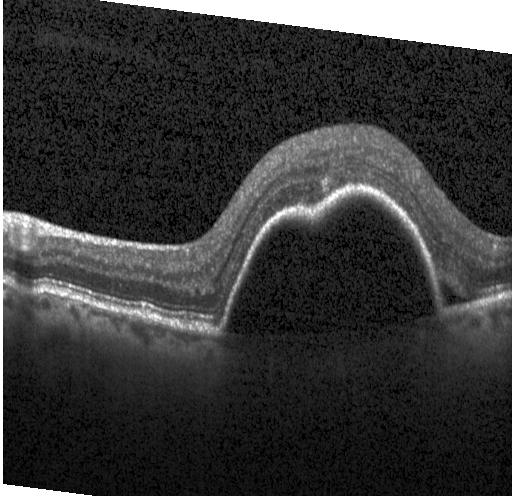 Optical coherence tomography scan
This B-scan demonstrates a choroidal neovascular membrane.